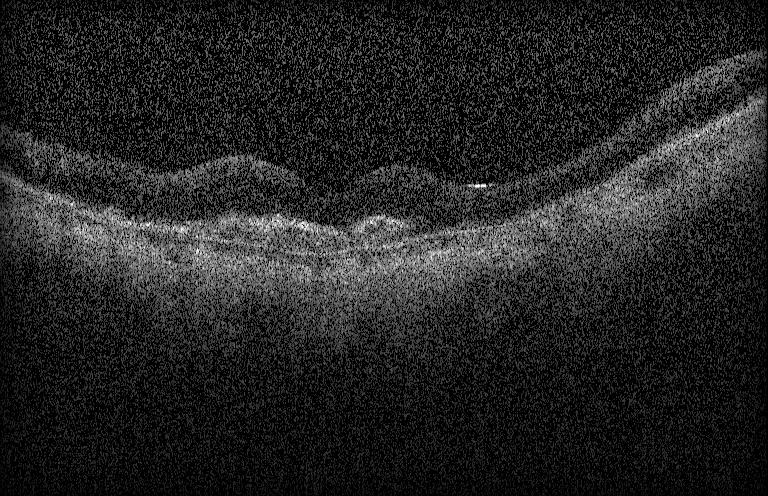

Macular OCT demonstrating choroidal neovascularization (CNV).